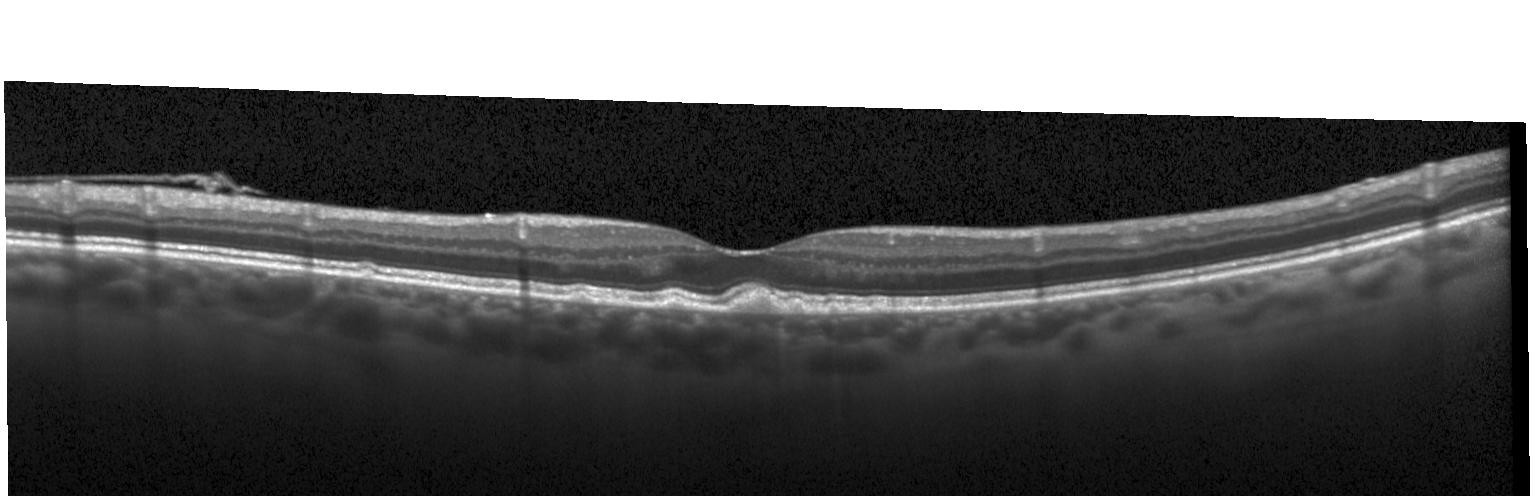
Retinal OCT cross-section showing drusen.